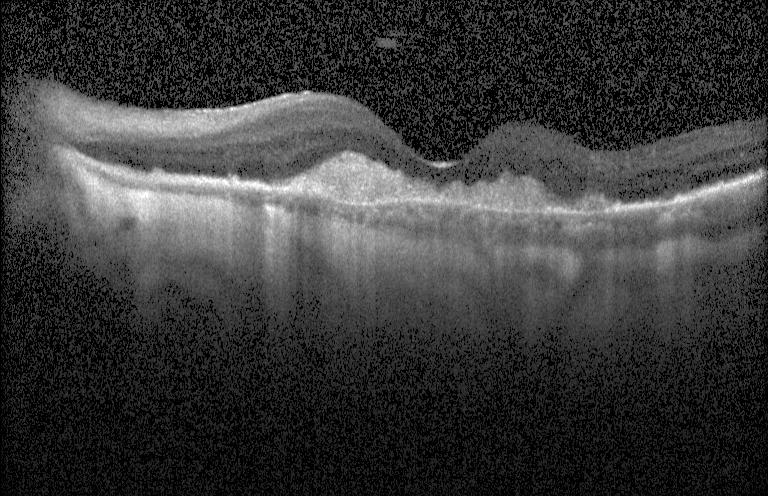
Acquired on a Heidelberg Spectralis. OCT B-scan. Spectral-domain OCT — This B-scan demonstrates choroidal neovascularization.